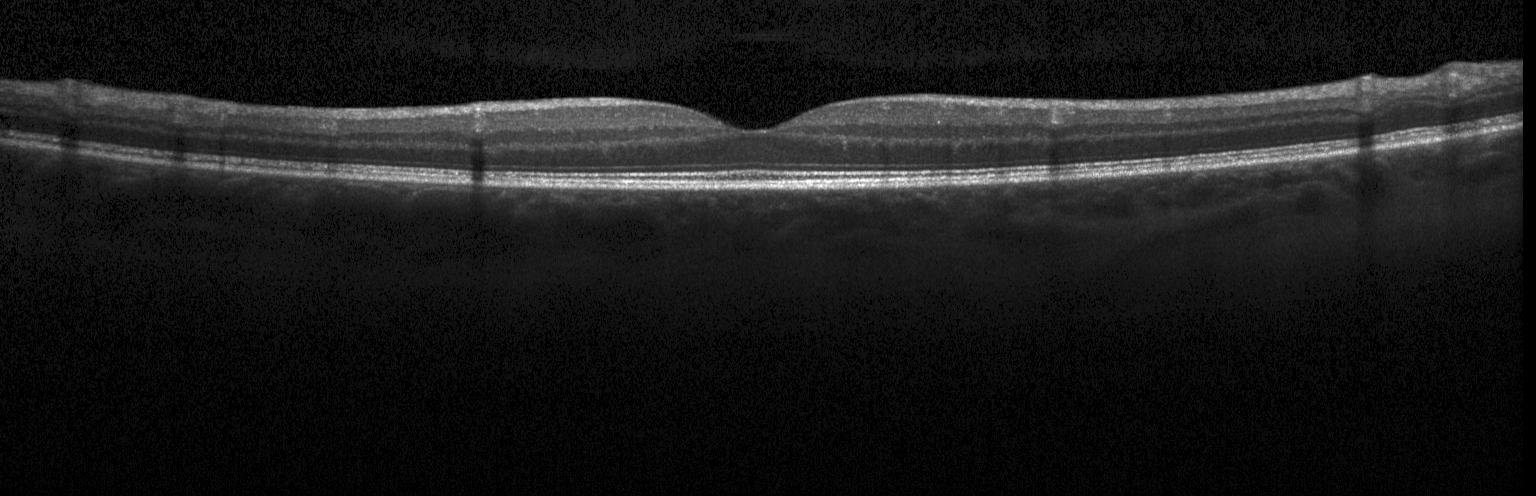
Retinal OCT cross-section showing neither CNV, DME, nor drusen.